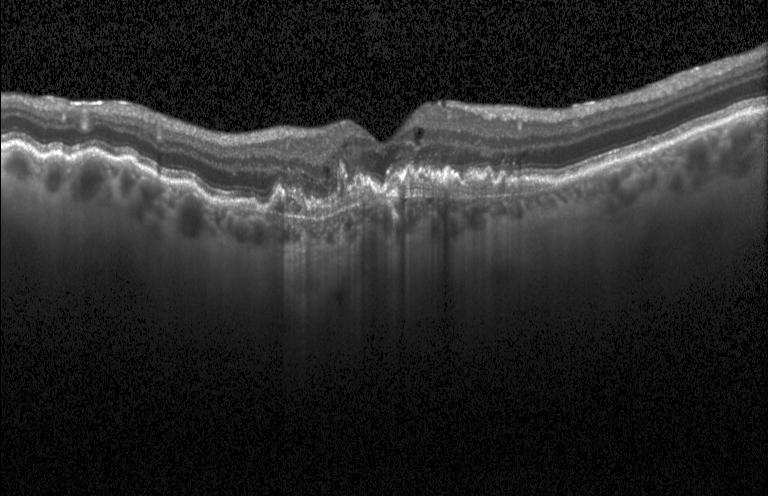 OCT line scan — Impression: CNV.